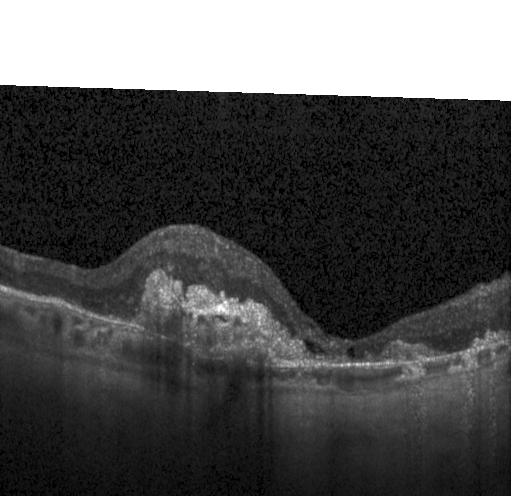

Finding: a choroidal neovascular membrane.